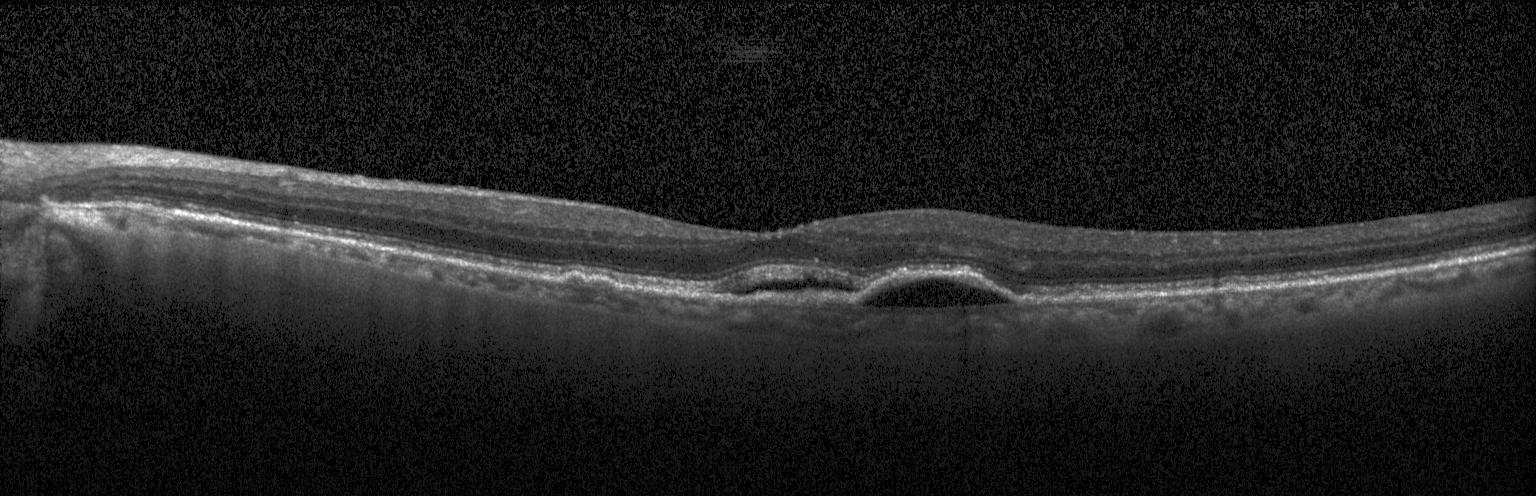

Optical coherence tomography scan, Heidelberg Spectralis, macular scan. Dx: a choroidal neovascular membrane.